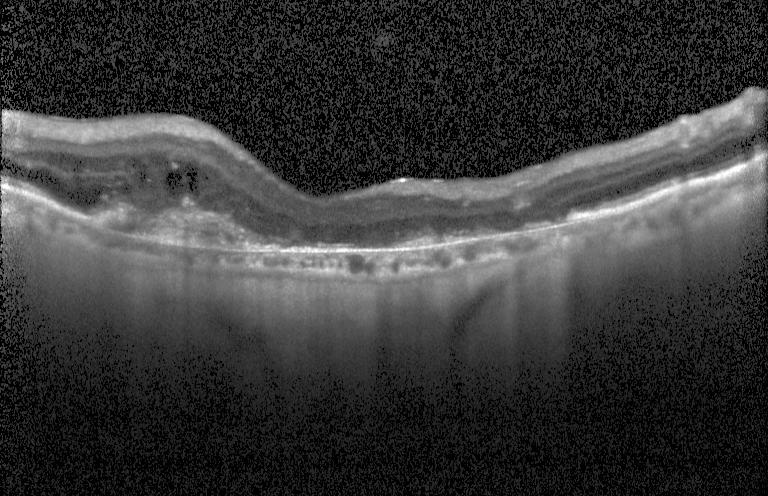

Dx: a choroidal neovascular membrane.